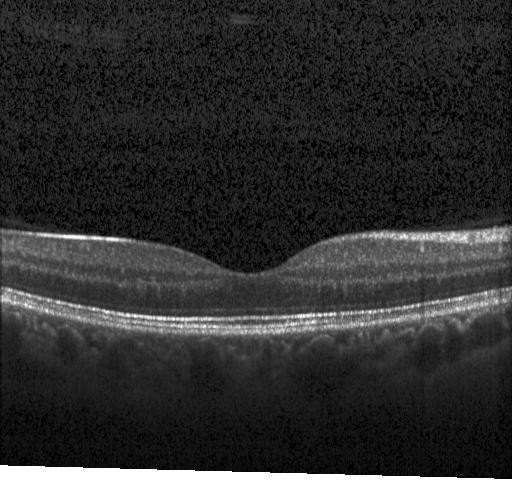 Retinal OCT B-scan · centered on the fovea — This B-scan demonstrates no choroidal neovascularization, no diabetic macular edema, and no drusen.